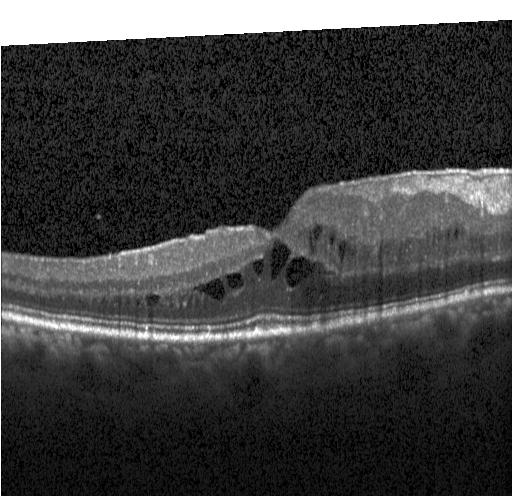 Optical coherence tomography B-scan
Impression: diabetic macular edema.